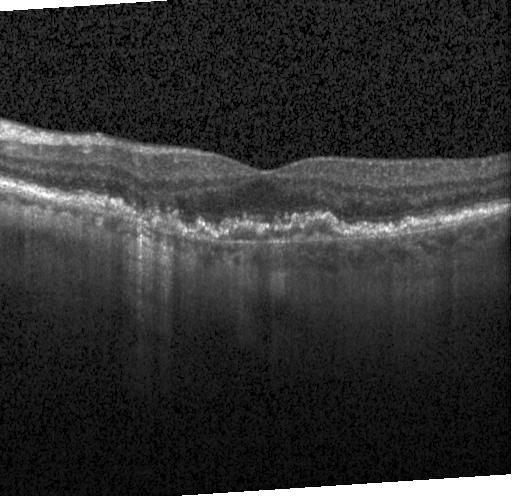
OCT line scan · through the macula · spectral-domain OCT.
Finding: CNV.